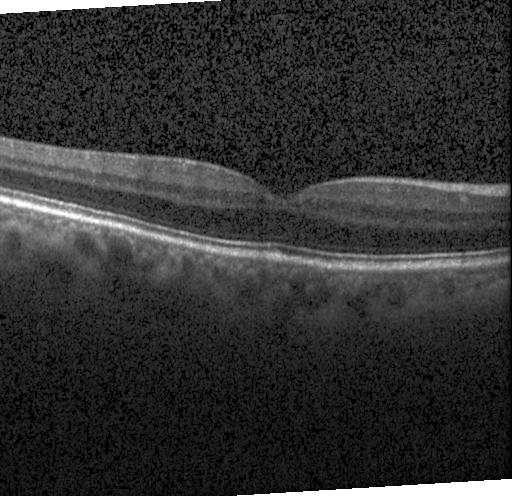 Optical coherence tomography scan. Through the macula. This B-scan demonstrates no choroidal neovascularization, diabetic macular edema, or drusen.